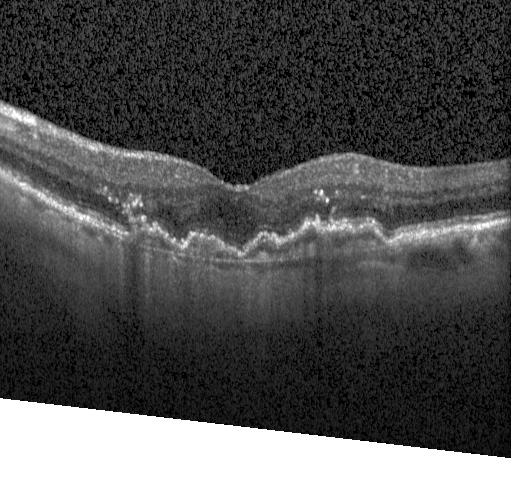
Heidelberg Spectralis OCT system; optical coherence tomography B-scan; spectral-domain OCT; centered on the fovea
Impression: CNV.